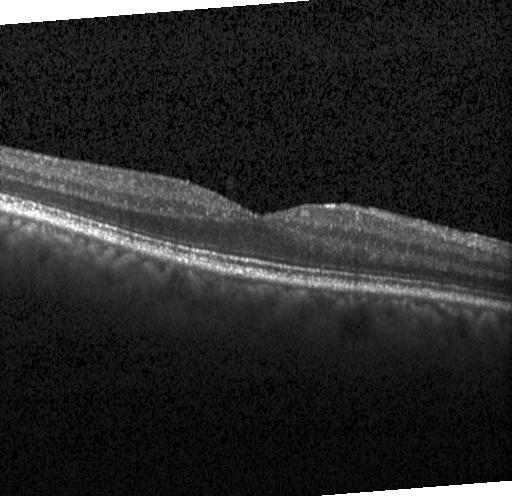

Impression: no evidence of choroidal neovascularization, diabetic macular edema, or drusen.